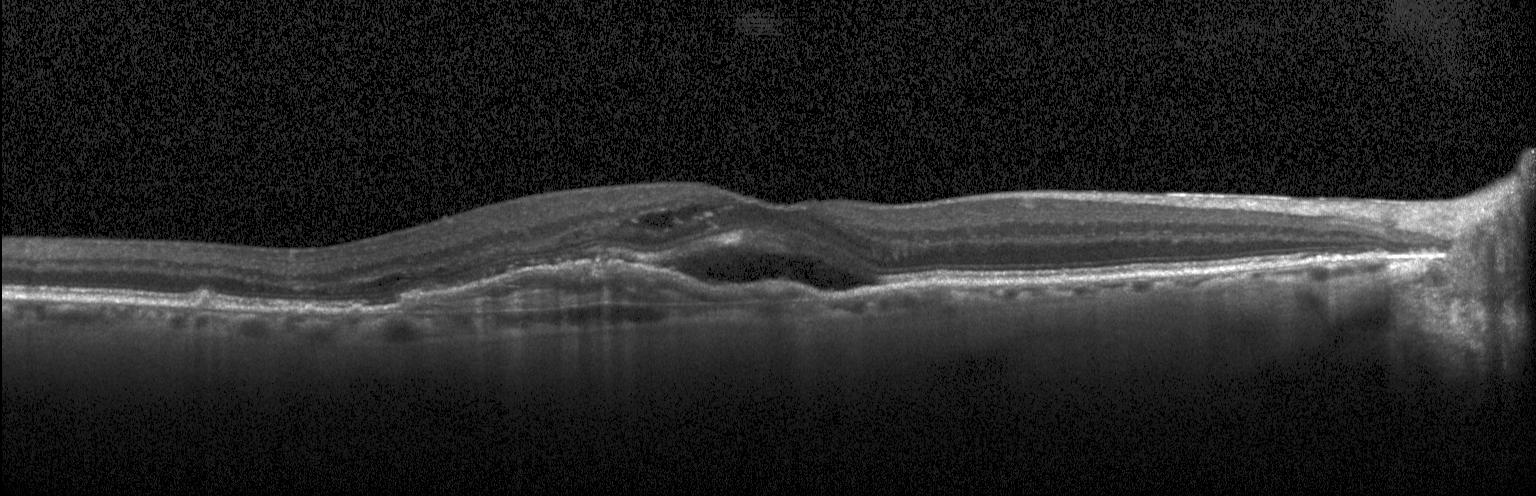

OCT line scan
The scan shows choroidal neovascularization.